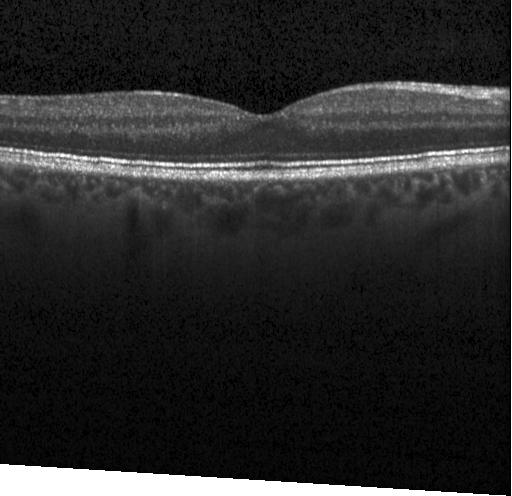
Optical coherence tomography scan. Acquired on a Heidelberg Spectralis. Impression: no choroidal neovascularization, diabetic macular edema, or drusen.